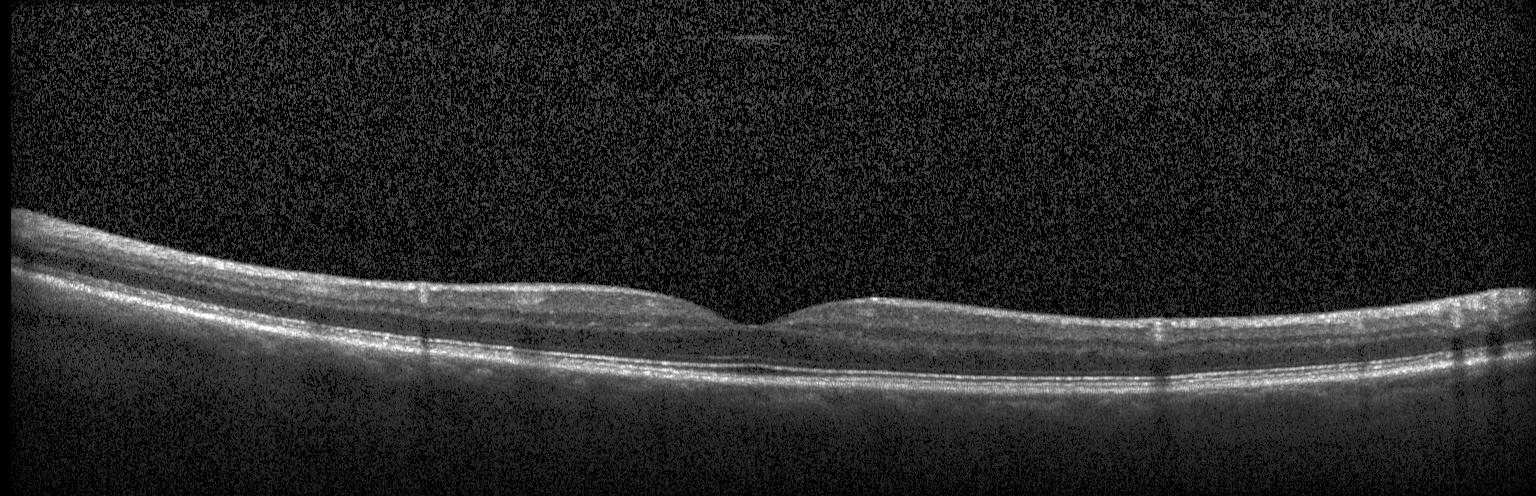

Retinal OCT B-scan
Diagnosis: neither choroidal neovascularization, diabetic macular edema, nor drusen.